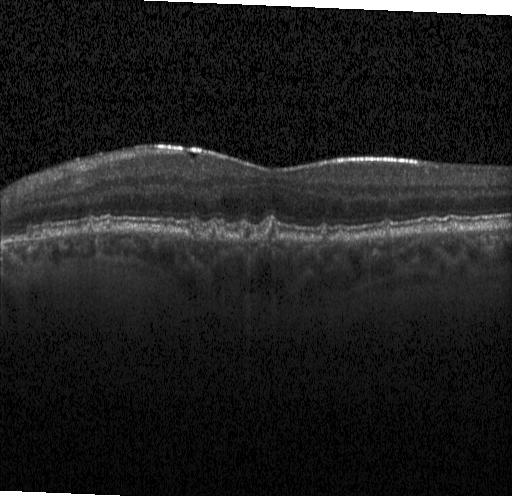
Spectral-domain optical coherence tomography · through the macula · instrument: Heidelberg Spectralis · optical coherence tomography scan — Diagnosis: drusen.